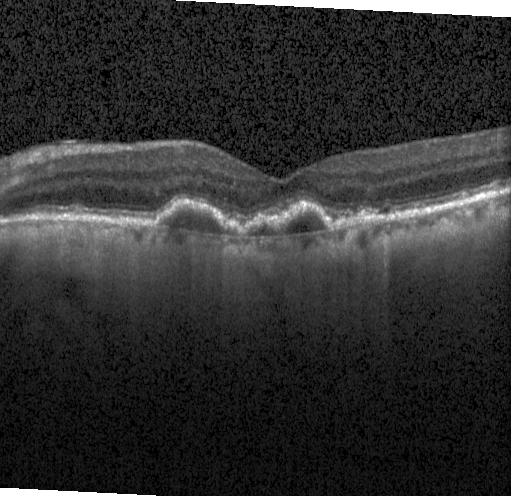 Spectral-domain optical coherence tomography · macular scan · optical coherence tomography scan · Heidelberg Spectralis — Diagnosis: CNV.